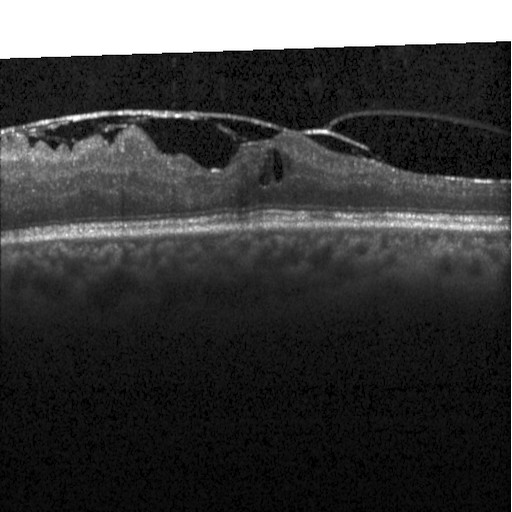 SD-OCT. Optical coherence tomography B-scan. Heidelberg Spectralis OCT system. Finding: diabetic macular edema (DME).